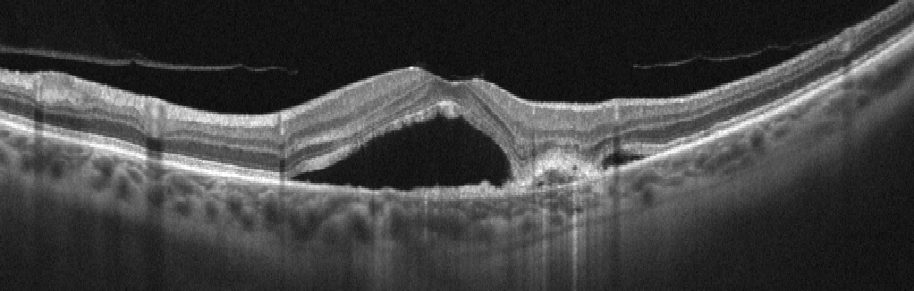
Instrument: Optovue Avanti RTVue XR. OCT line scan. Through the macula — The scan shows age-related macular degeneration (AMD).